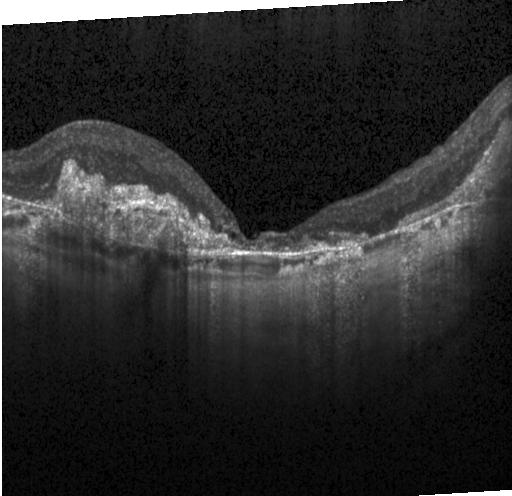

Retinal OCT cross-section. Choroidal neovascularization.